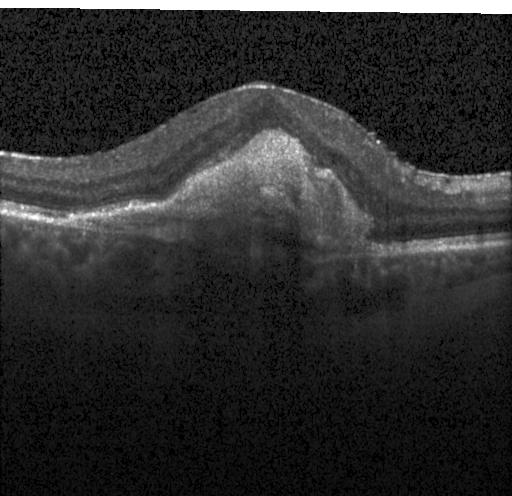

Finding: a choroidal neovascular membrane.